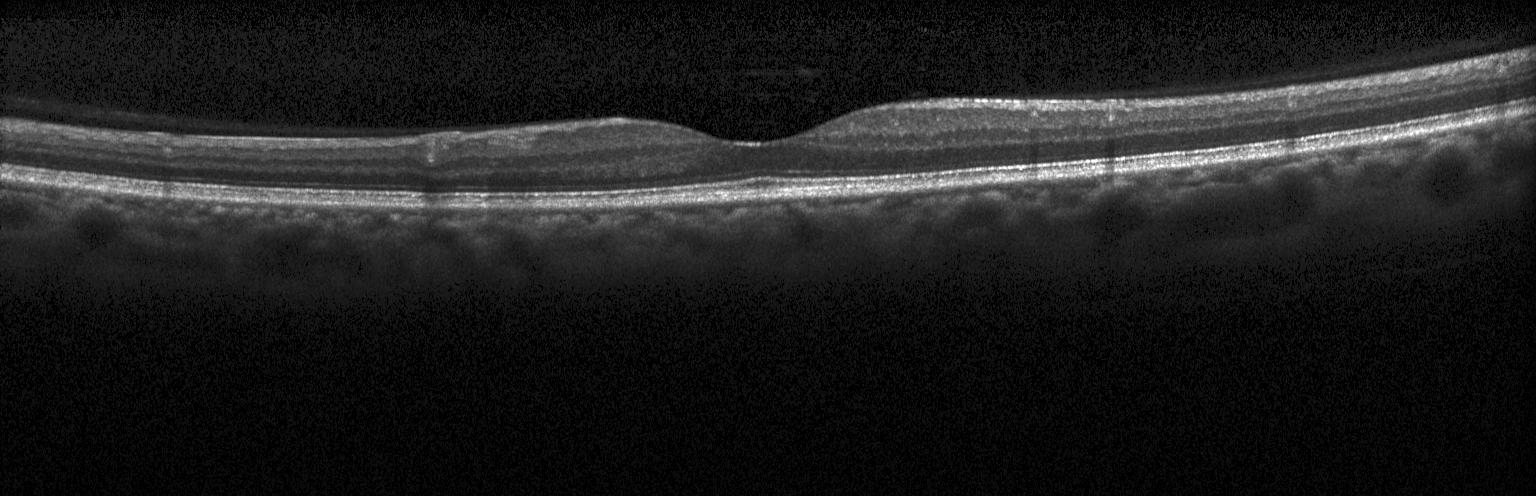 Optical coherence tomography B-scan
Diagnosis: no choroidal neovascularization, no diabetic macular edema, and no drusen.